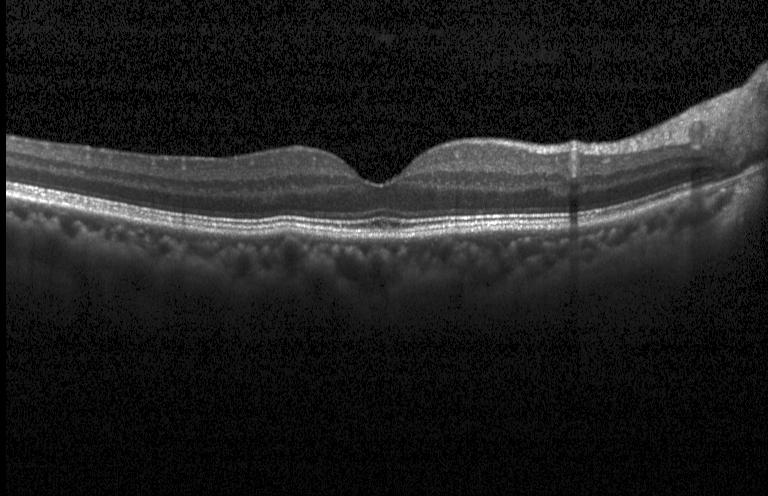

Spectral-domain OCT B-scan: no evidence of choroidal neovascularization, diabetic macular edema, or drusen.